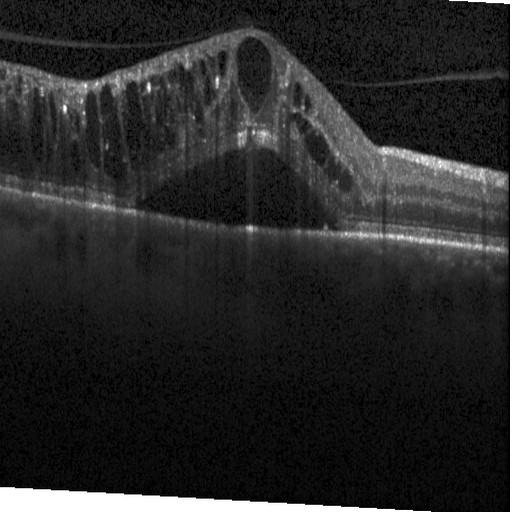
Dx: diabetic macular edema.